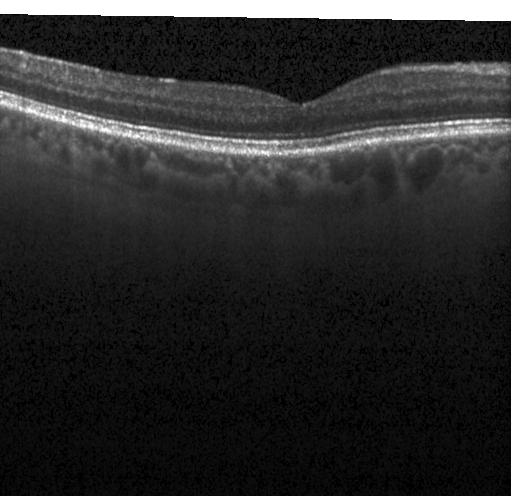 Optical coherence tomography scan. Centered on the fovea — Finding: no choroidal neovascularization, diabetic macular edema, or drusen.